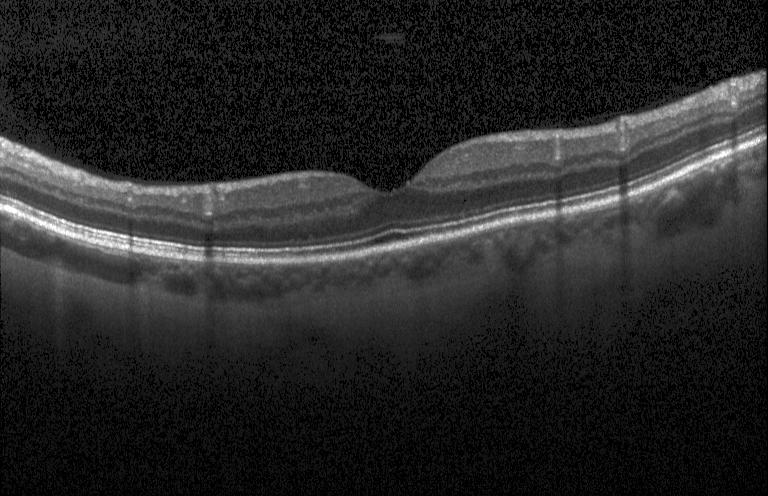 OCT finding: neither choroidal neovascularization, diabetic macular edema, nor drusen.